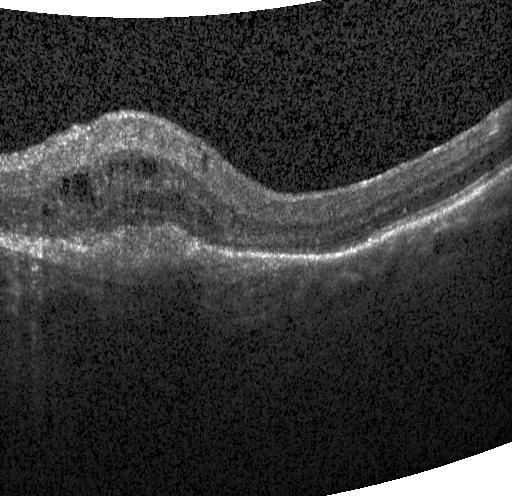
Centered on the fovea · OCT line scan · instrument: Heidelberg Spectralis — This B-scan demonstrates choroidal neovascularization (CNV).